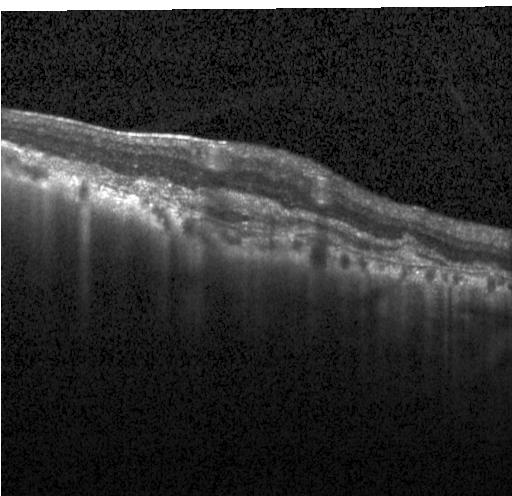
Diagnosis: choroidal neovascularization.